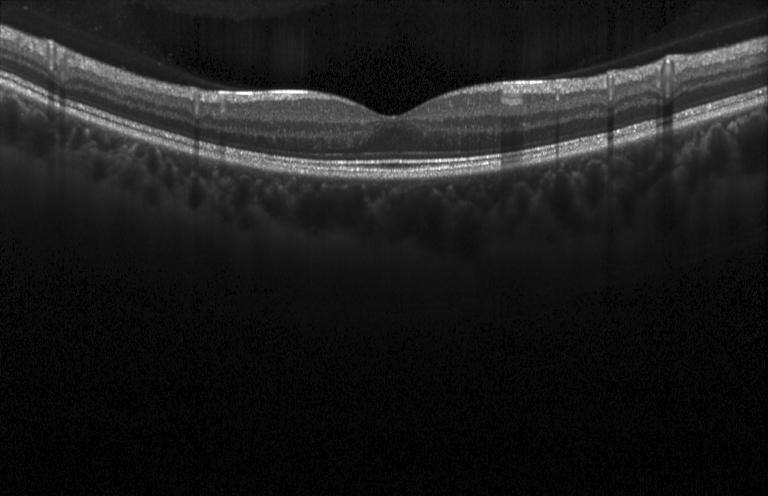 Diagnosis: no choroidal neovascularization, no diabetic macular edema, and no drusen.